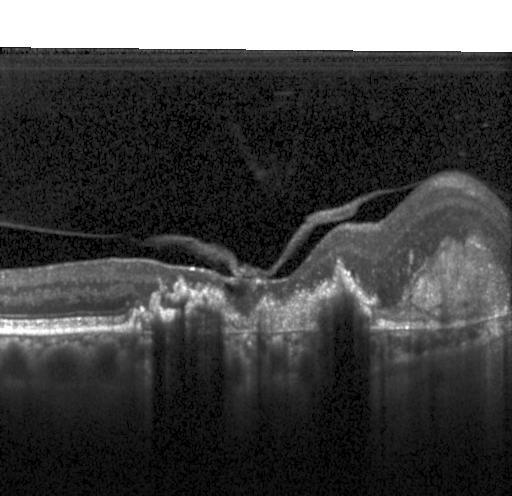
Impression: choroidal neovascularization (CNV).